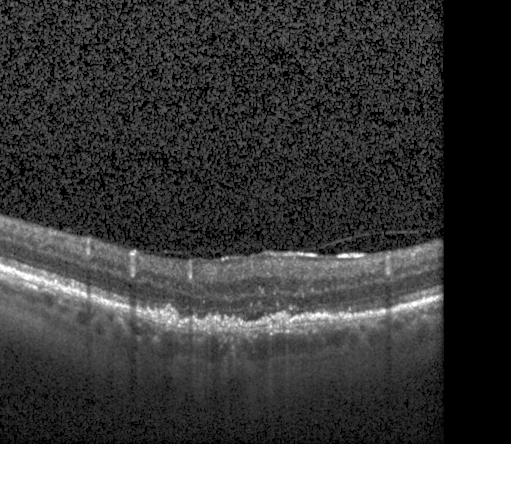

OCT B-scan
Macular OCT: a choroidal neovascular membrane.